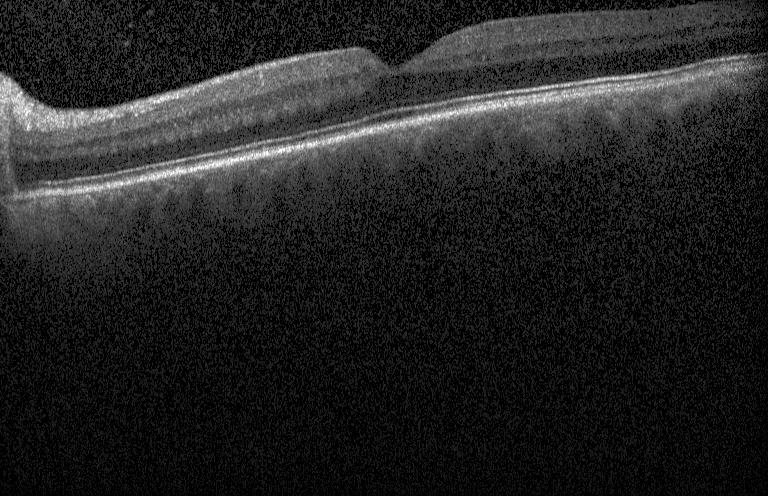 Retinal OCT cross-section, Heidelberg Spectralis OCT system, horizontal scan through the fovea.
No evidence of CNV, DME, or drusen.